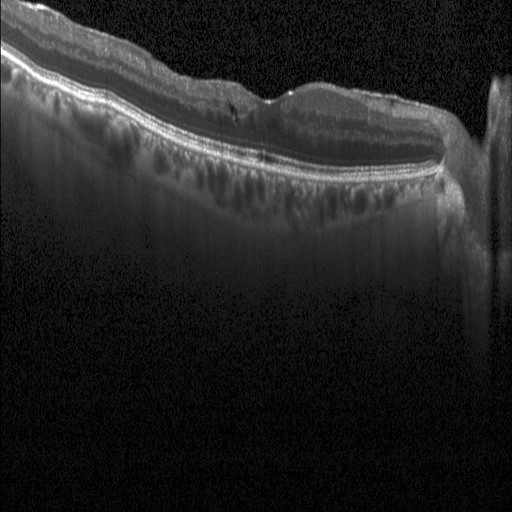 OCT line scan. Macular scan. SD-OCT. Acquired on a Heidelberg Spectralis.
OCT finding: diabetic macular edema (DME).